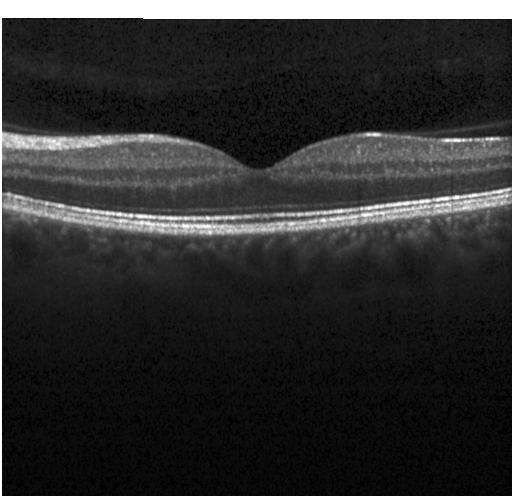 Acquired on a Heidelberg Spectralis. Spectral-domain optical coherence tomography. Macular scan. OCT line scan — This B-scan demonstrates no evidence of CNV, DME, or drusen.